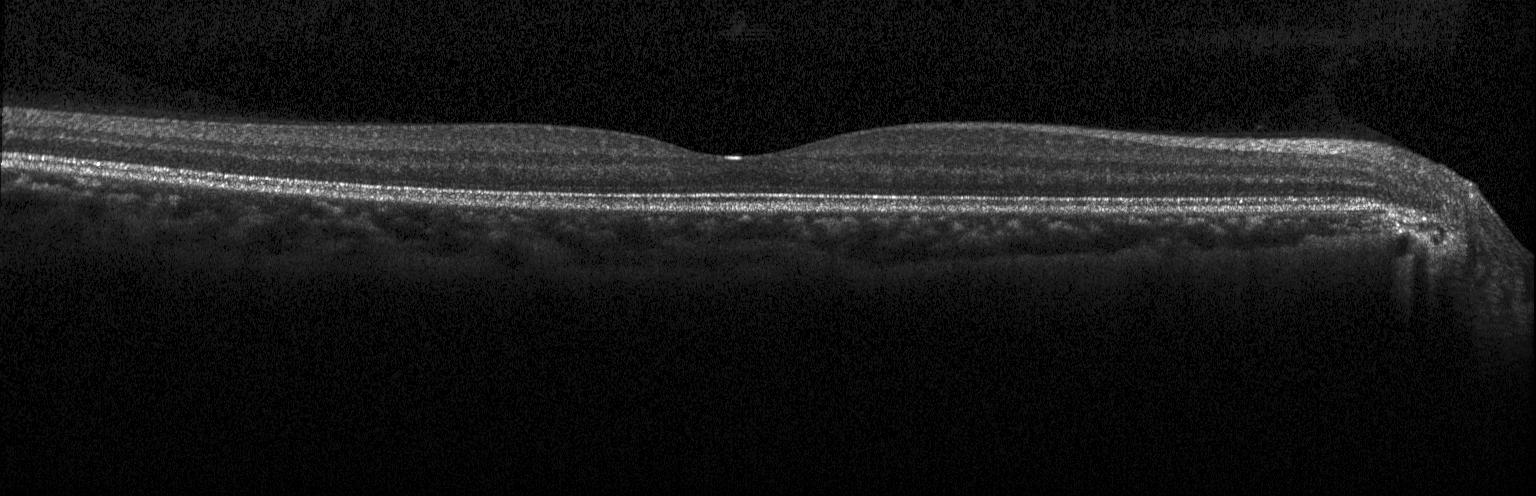 Finding: neither CNV, DME, nor drusen.